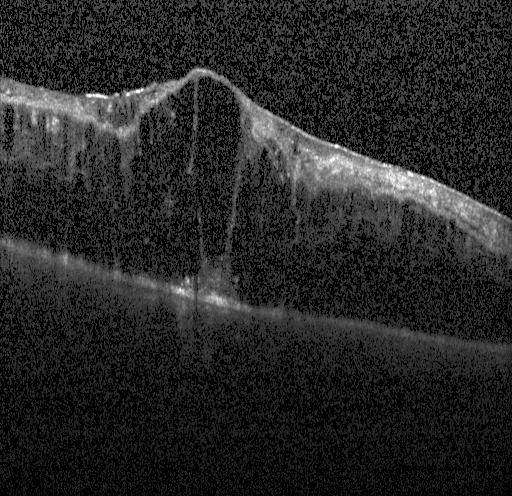
Through the macula; optical coherence tomography B-scan. The scan shows diabetic macular edema (DME).